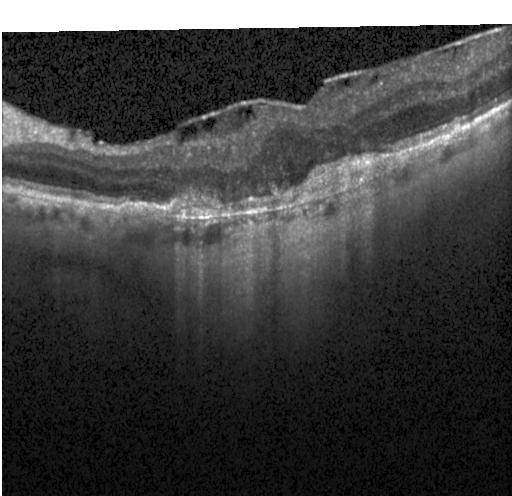
Diagnosis: a choroidal neovascular membrane.